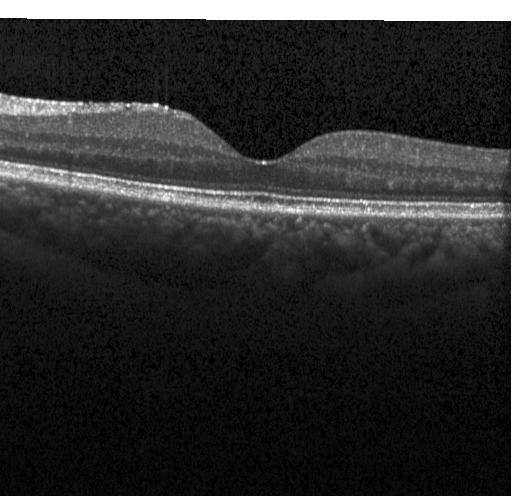

Macular scan. Spectral-domain optical coherence tomography. Retinal OCT B-scan
Diagnosis: no CNV, no DME, and no drusen.